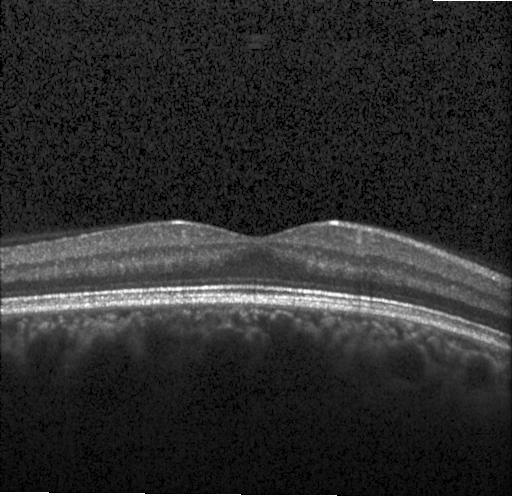
Impression: no choroidal neovascularization, diabetic macular edema, or drusen.